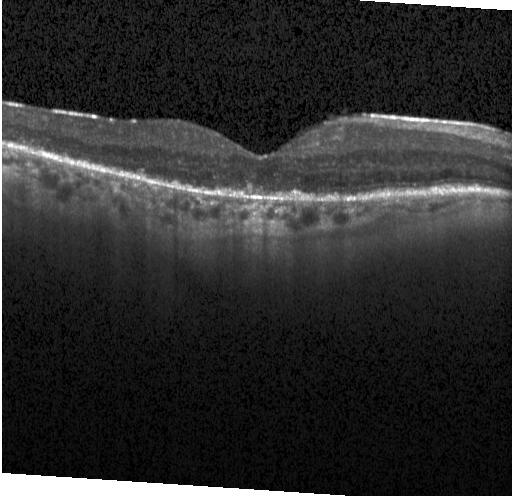

Impression: neither choroidal neovascularization, diabetic macular edema, nor drusen.